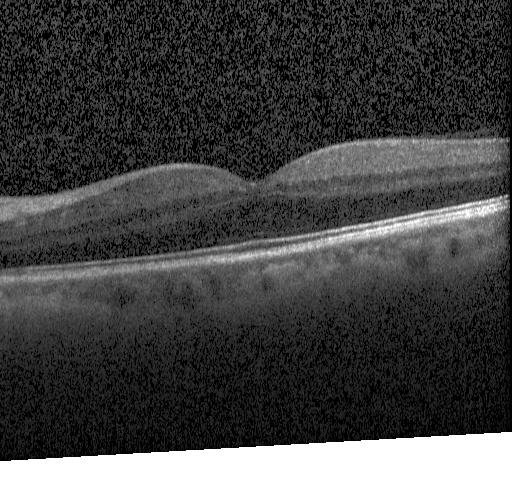 Optical coherence tomography scan.
Macular OCT: no choroidal neovascularization, diabetic macular edema, or drusen.